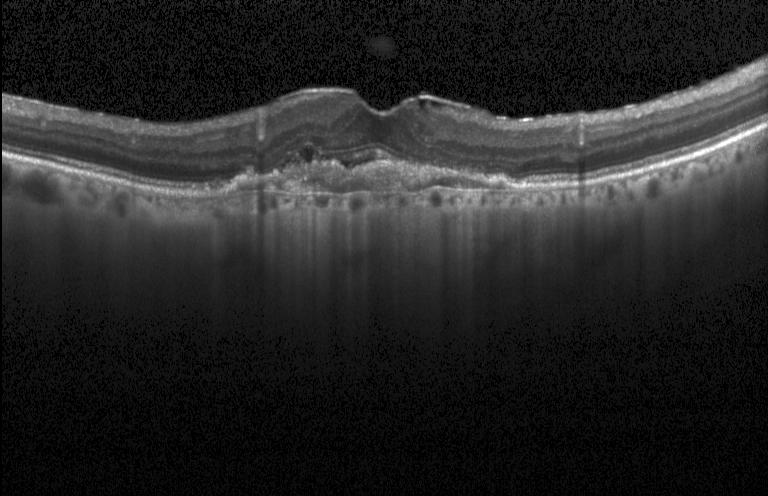
Acquired on a Heidelberg Spectralis. OCT line scan
This B-scan demonstrates a choroidal neovascular membrane.